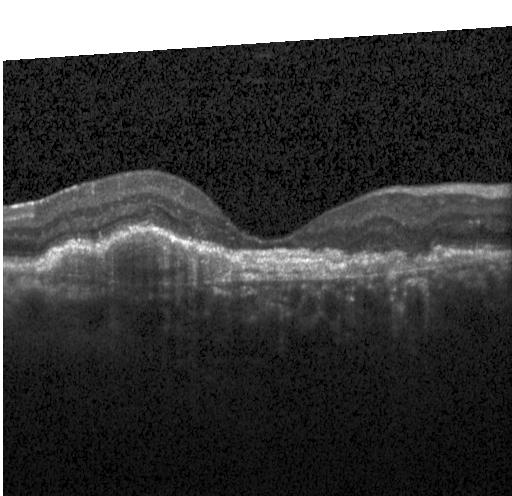
Impression: a choroidal neovascular membrane.